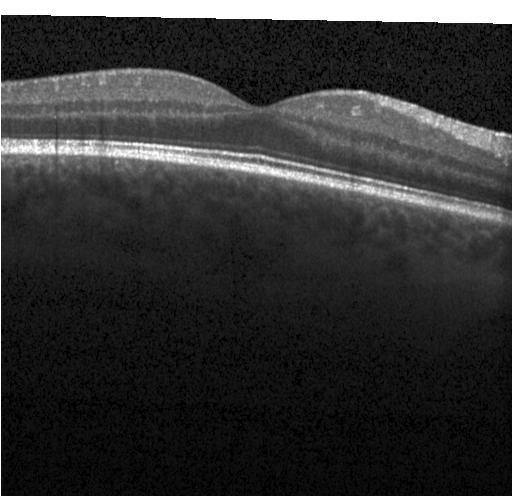

Macular scan. Spectral-domain optical coherence tomography. Optical coherence tomography B-scan.
Finding: no CNV, no DME, and no drusen.